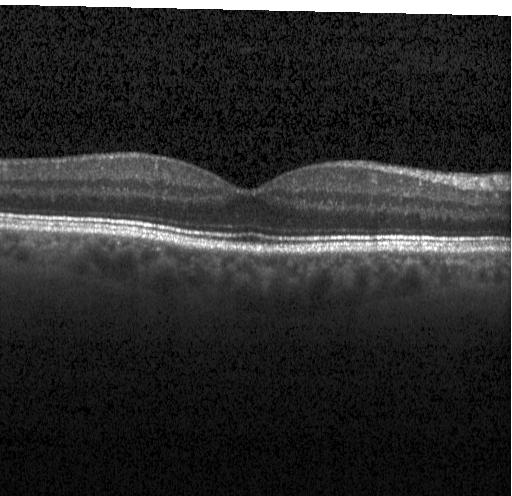

Heidelberg Spectralis; fovea-centered; optical coherence tomography B-scan — Finding: no choroidal neovascularization, no diabetic macular edema, and no drusen.